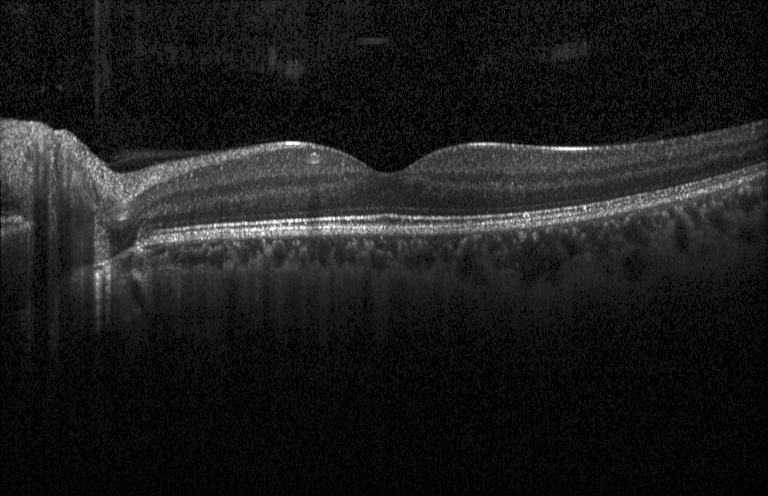
Retinal OCT cross-section showing no choroidal neovascularization, no diabetic macular edema, and no drusen.